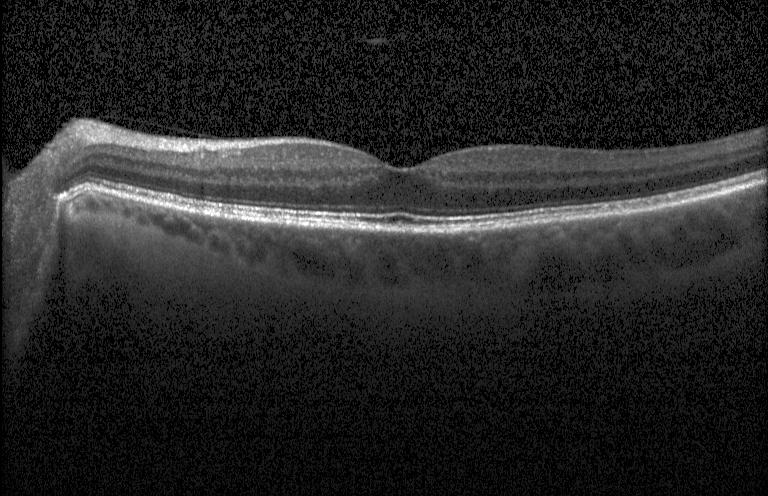
Macular OCT demonstrating no choroidal neovascularization, diabetic macular edema, or drusen.